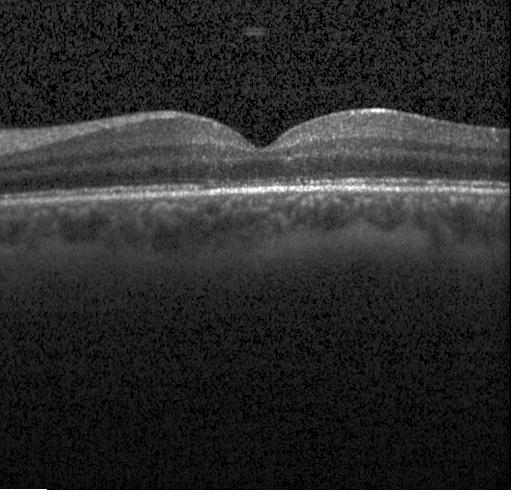

OCT B-scan. Centered on the fovea.
Impression: no evidence of choroidal neovascularization, diabetic macular edema, or drusen.